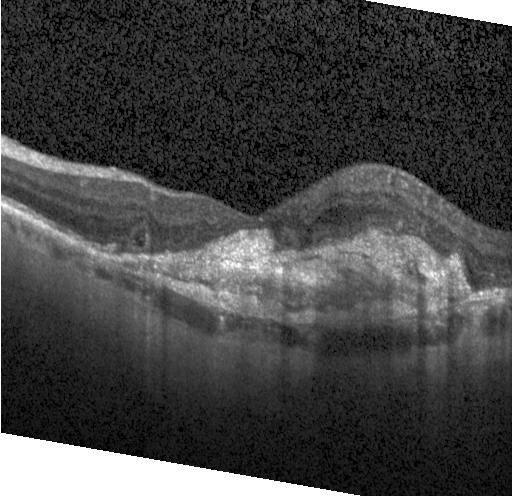

Diagnosis: a choroidal neovascular membrane.